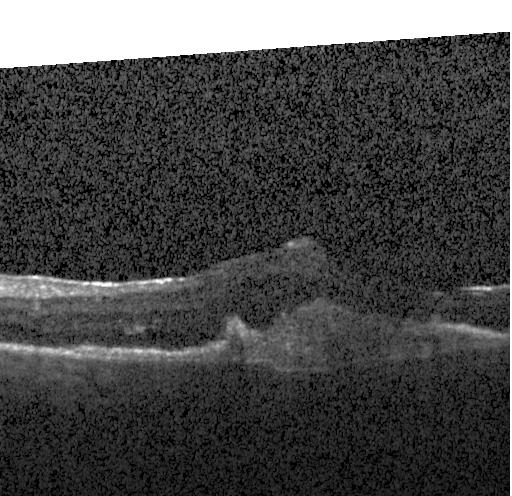
Retinal OCT cross-section
Assessment: a choroidal neovascular membrane.